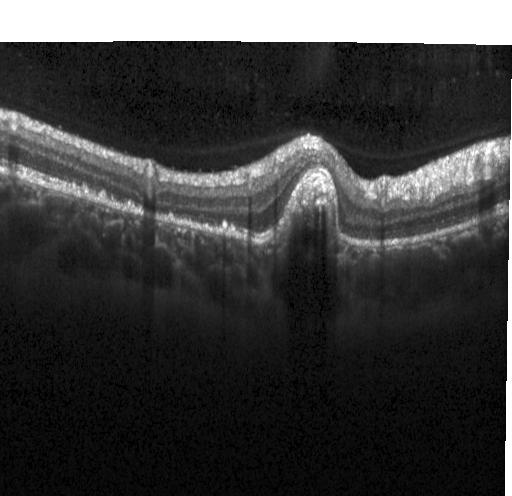
Acquired on a Heidelberg Spectralis; SD-OCT; horizontal scan through the fovea; OCT B-scan.
Assessment: a choroidal neovascular membrane.